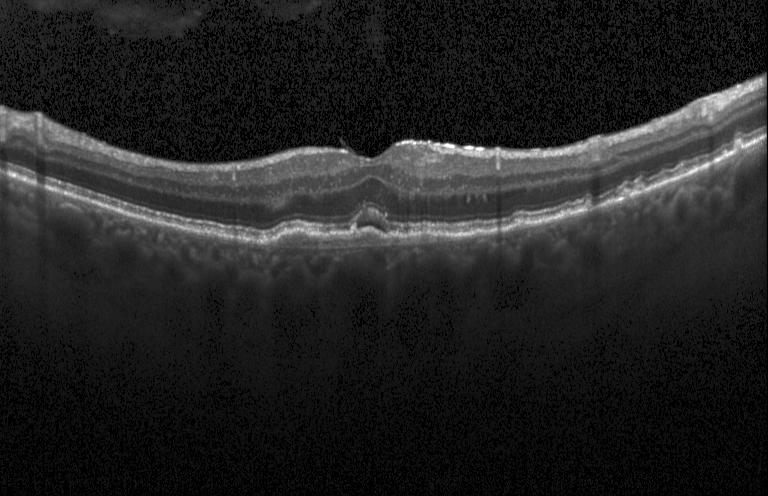
Optical coherence tomography scan. Spectral-domain optical coherence tomography
This B-scan demonstrates CNV.